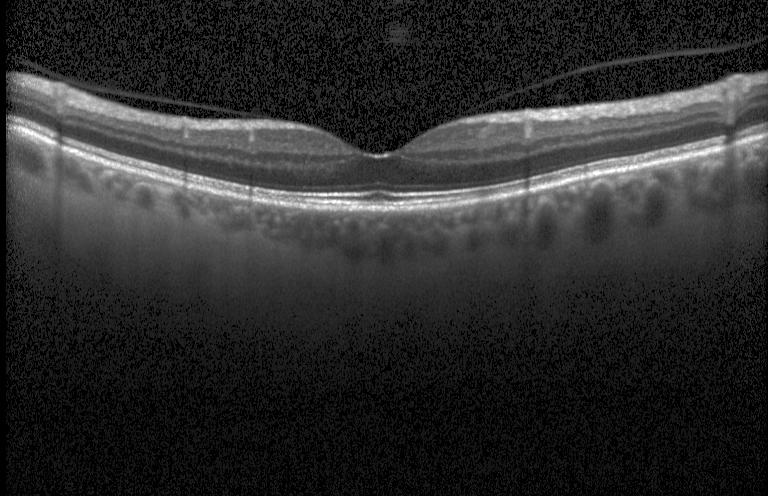 Acquired on a Heidelberg Spectralis. Macular scan. OCT B-scan. Spectral-domain optical coherence tomography.
Assessment: no evidence of CNV, DME, or drusen.